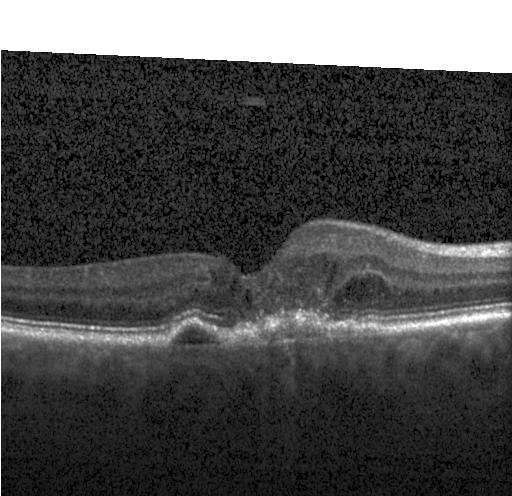
Macular scan. OCT line scan
Assessment: a choroidal neovascular membrane.